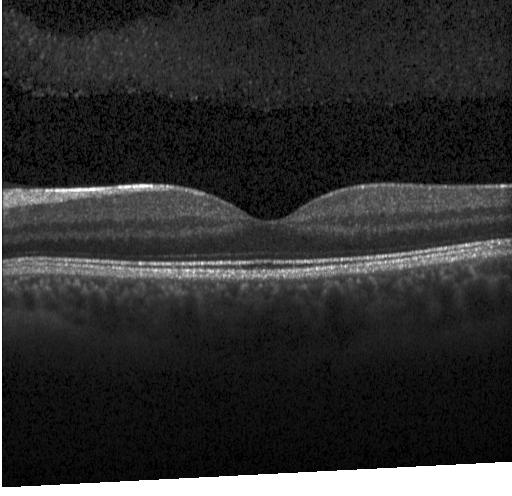
OCT B-scan — Diagnosis: no choroidal neovascularization, diabetic macular edema, or drusen.